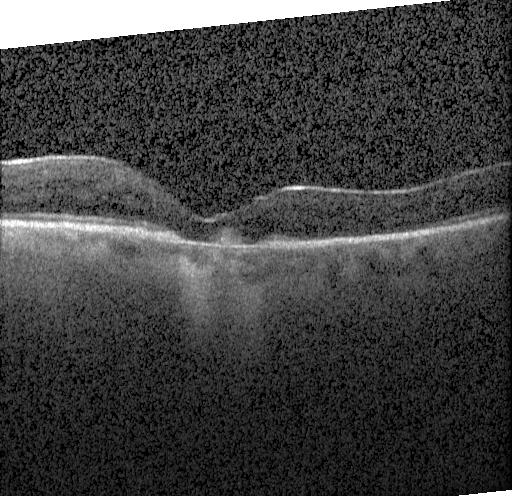
OCT finding: choroidal neovascularization.